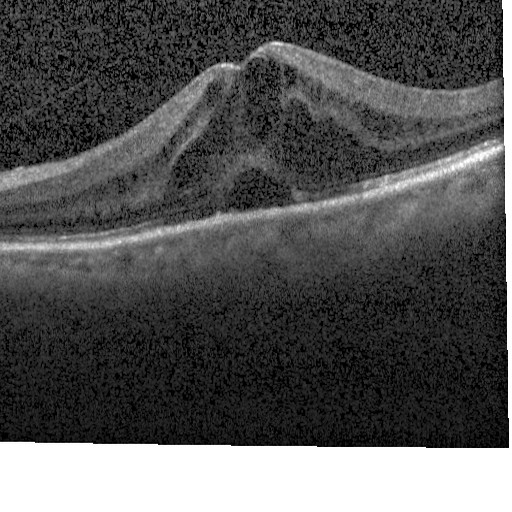

The scan shows diabetic macular edema (DME).